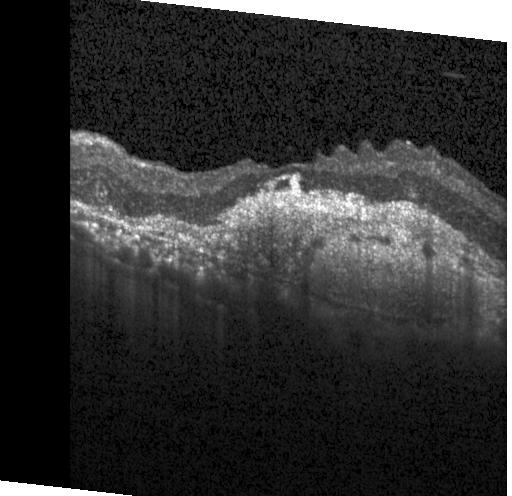
Retinal OCT B-scan. Instrument: Heidelberg Spectralis — CNV.